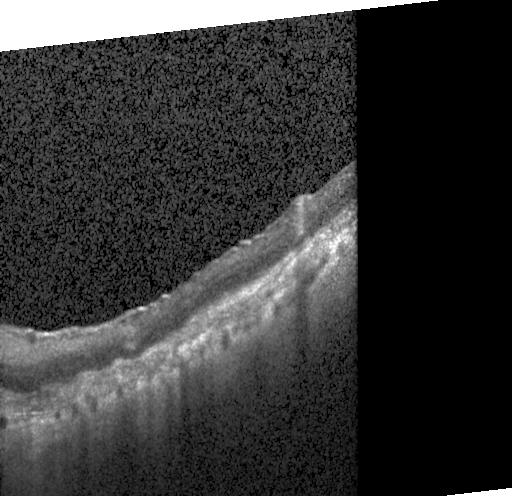
SD-OCT; retinal OCT cross-section; horizontal scan through the fovea; Heidelberg Spectralis OCT system
Choroidal neovascularization (CNV).